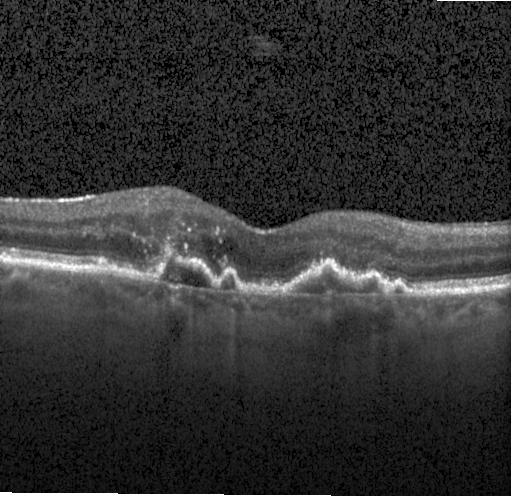
OCT finding: choroidal neovascularization.